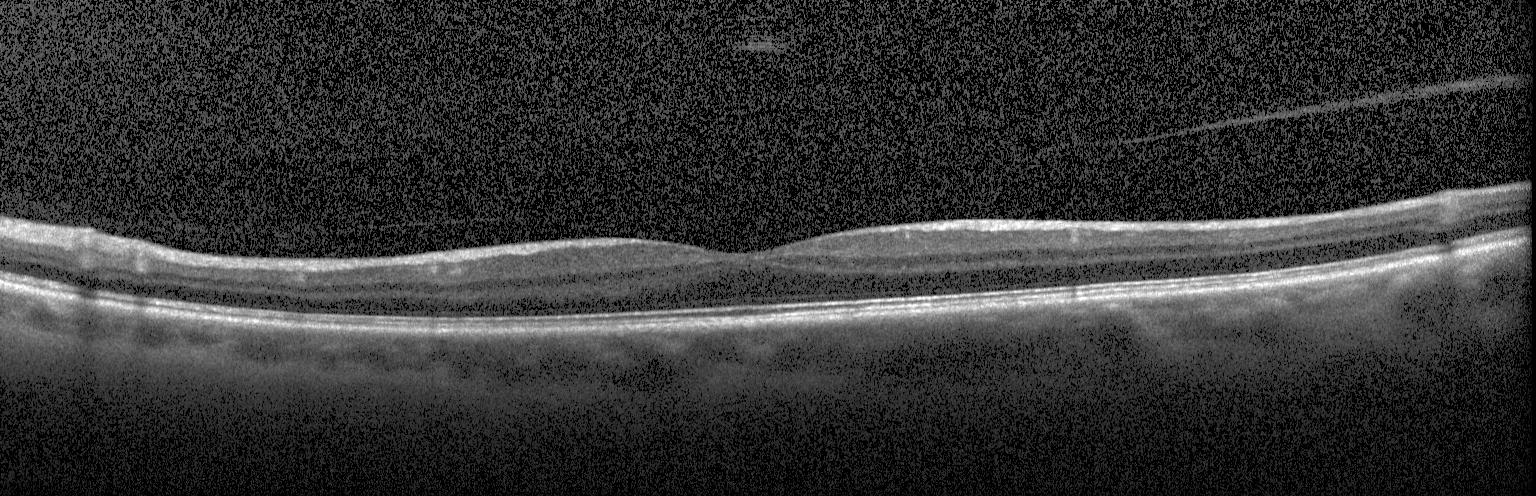
OCT scan showing no choroidal neovascularization, no diabetic macular edema, and no drusen.